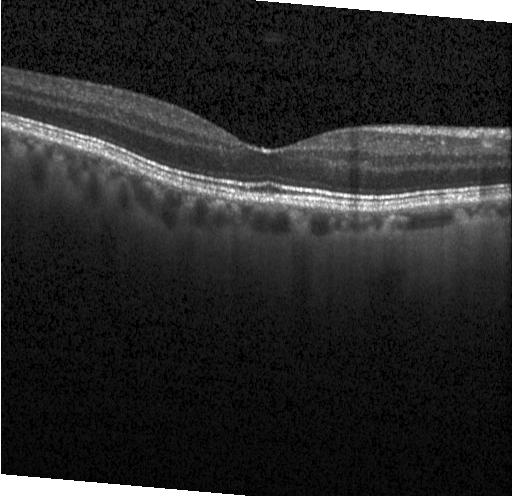 Retinal OCT B-scan
Impression: no choroidal neovascularization, diabetic macular edema, or drusen.